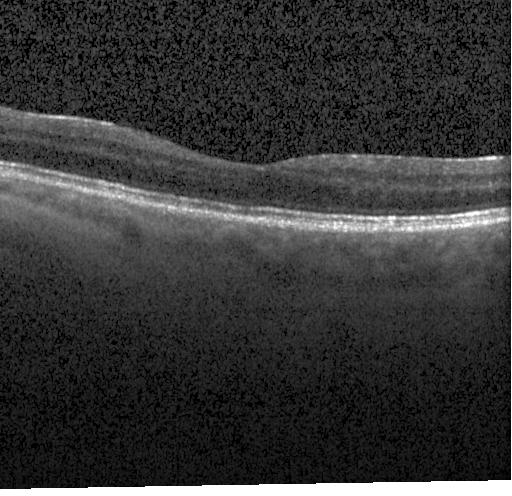

Optical coherence tomography scan, spectral-domain OCT — Macular OCT: no choroidal neovascularization, diabetic macular edema, or drusen.